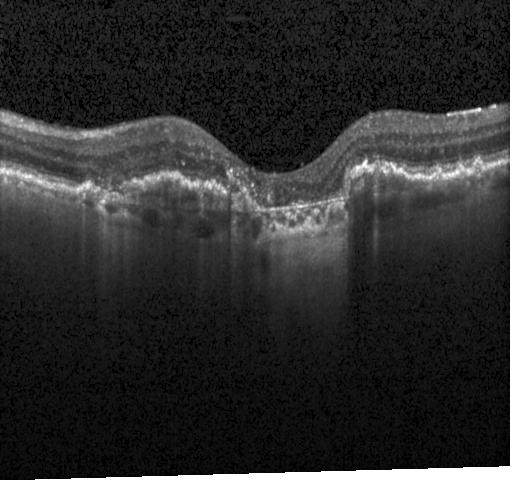 Retinal OCT cross-section. This B-scan demonstrates CNV.